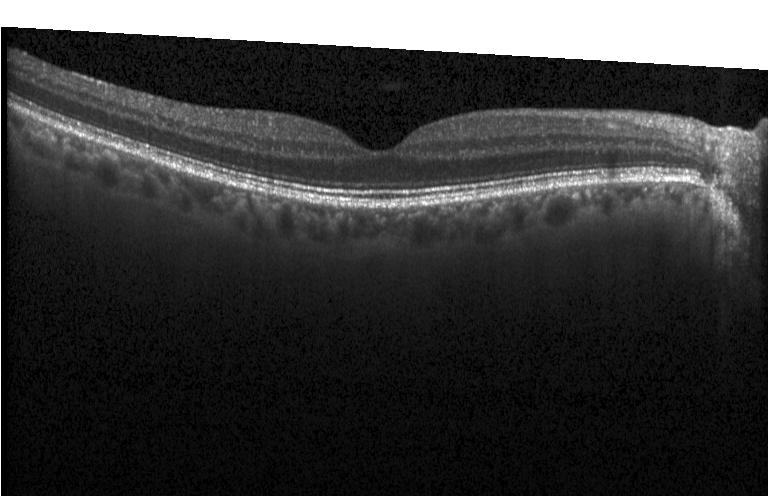 Assessment: no evidence of choroidal neovascularization, diabetic macular edema, or drusen.